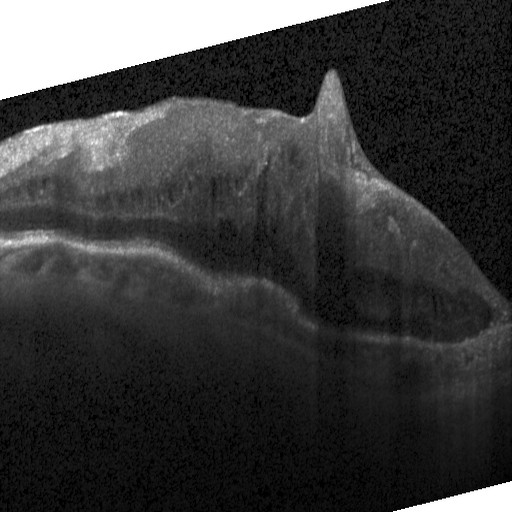

Fovea-centered; optical coherence tomography B-scan; acquired on a Heidelberg Spectralis. Assessment: diabetic macular edema (DME).